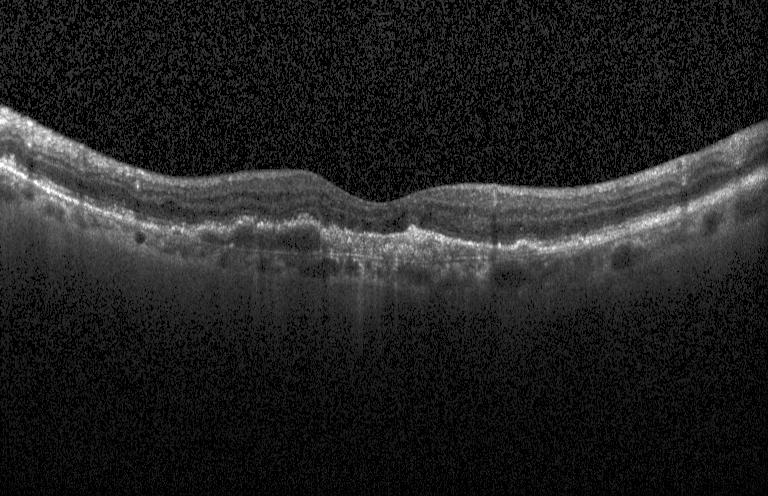 Optical coherence tomography scan. A choroidal neovascular membrane.